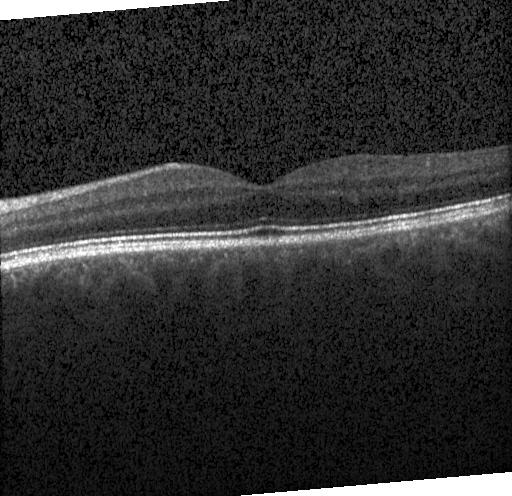
Retinal OCT cross-section — Finding: neither choroidal neovascularization, diabetic macular edema, nor drusen.